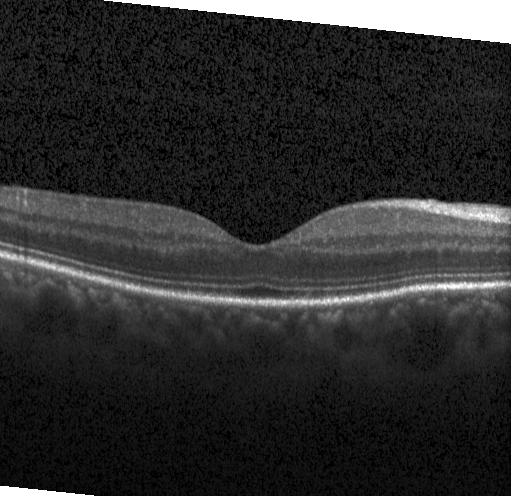 Spectral-domain OCT · OCT line scan — Finding: no CNV, no DME, and no drusen.